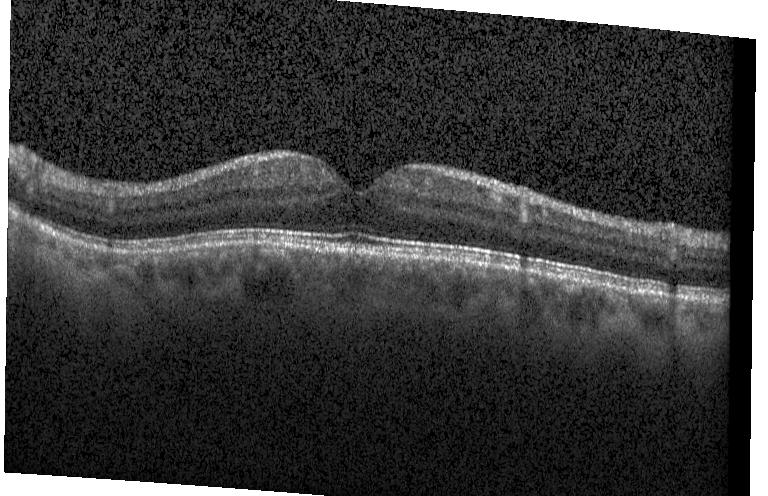

Impression: no choroidal neovascularization, diabetic macular edema, or drusen.